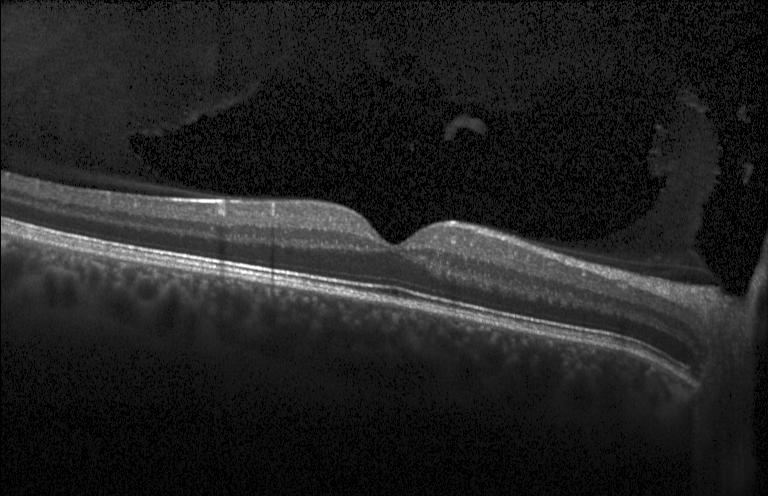
Heidelberg Spectralis; SD-OCT; optical coherence tomography B-scan; fovea-centered
This B-scan demonstrates no choroidal neovascularization, no diabetic macular edema, and no drusen.